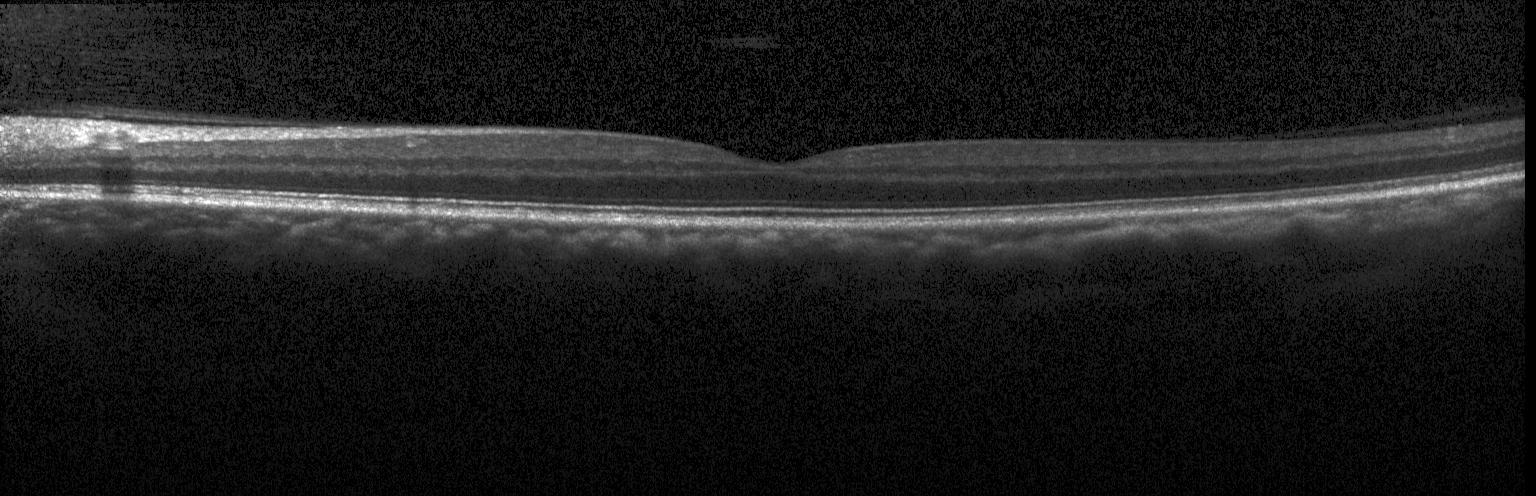 Diagnosis: no choroidal neovascularization, diabetic macular edema, or drusen.